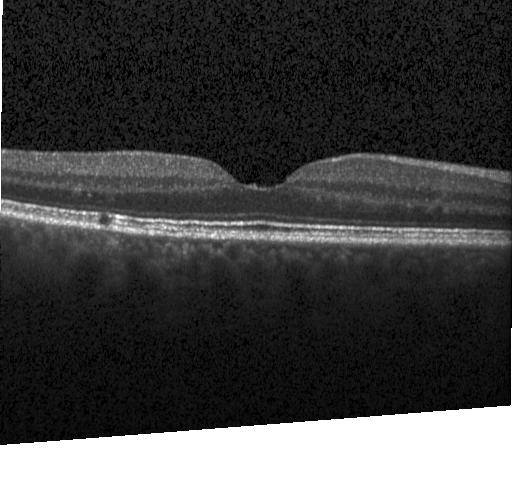 Centered on the fovea; SD-OCT; instrument: Heidelberg Spectralis; optical coherence tomography B-scan. Dx: no choroidal neovascularization, no diabetic macular edema, and no drusen.